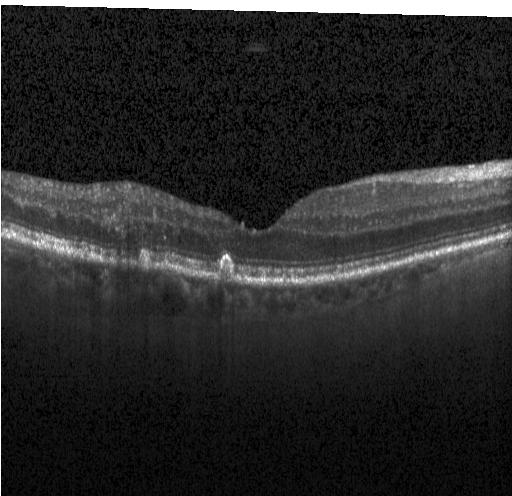 Macular OCT demonstrating drusen.